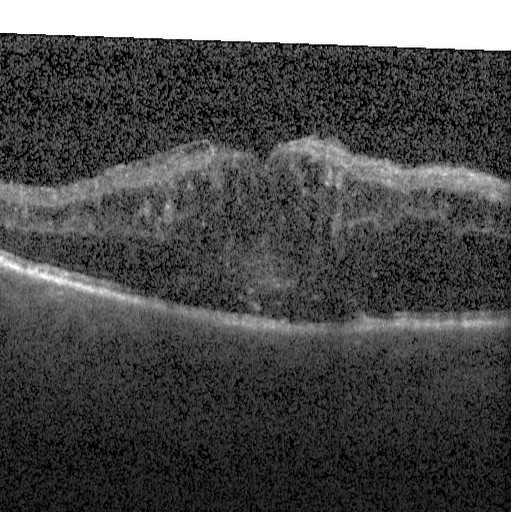

The scan shows DME.